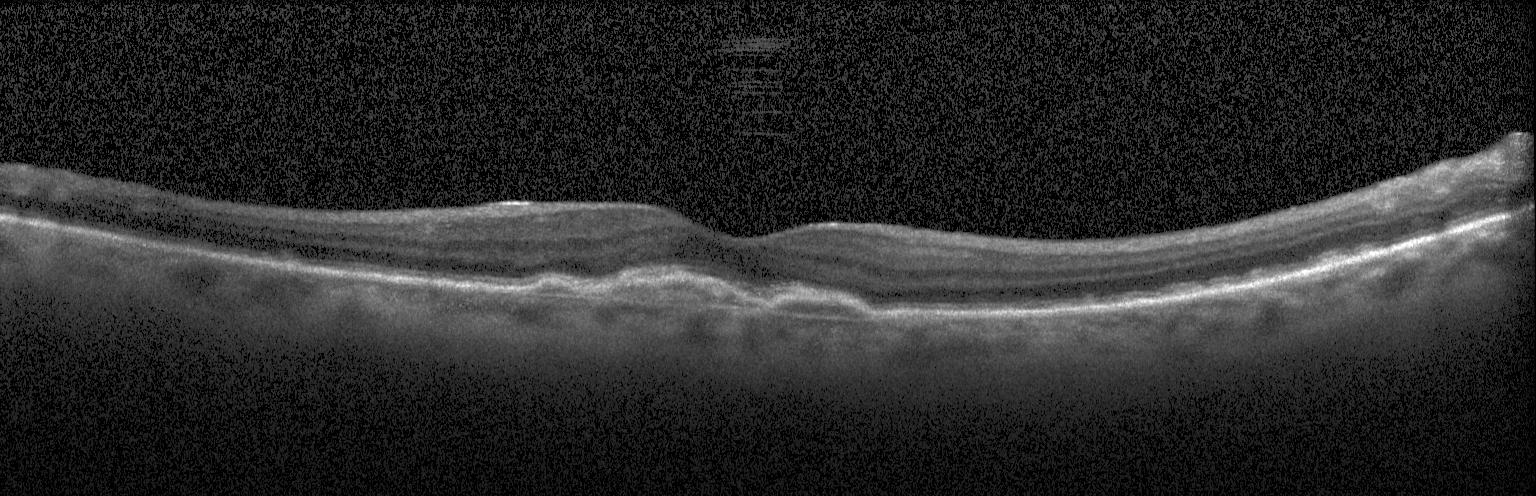
OCT B-scan. Macular OCT: a choroidal neovascular membrane.